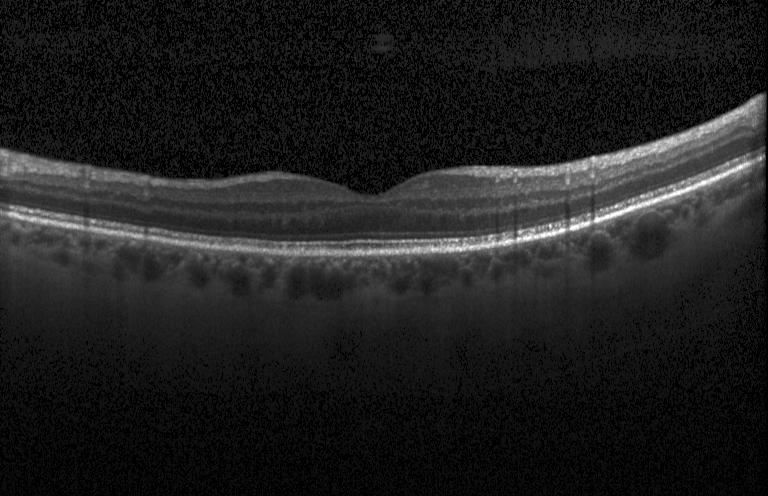 OCT line scan, SD-OCT — Diagnosis: no evidence of choroidal neovascularization, diabetic macular edema, or drusen.